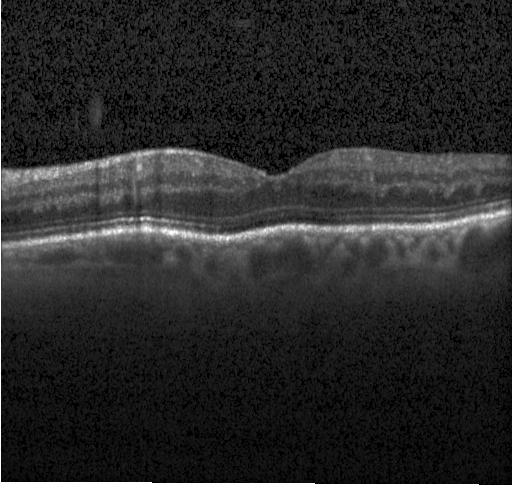
Optical coherence tomography B-scan. Heidelberg Spectralis
Diagnosis: no evidence of choroidal neovascularization, diabetic macular edema, or drusen.